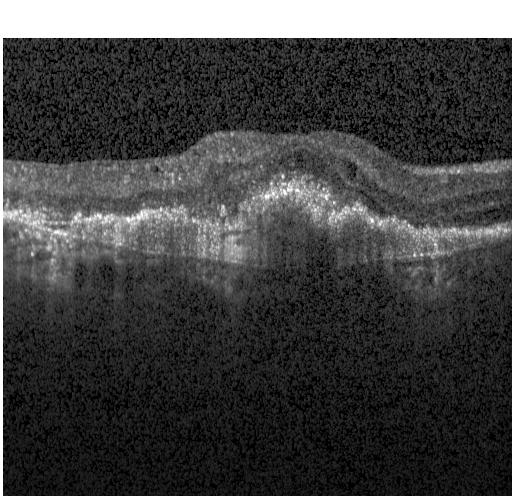 Through the macula, optical coherence tomography scan, spectral-domain OCT
The scan shows CNV.